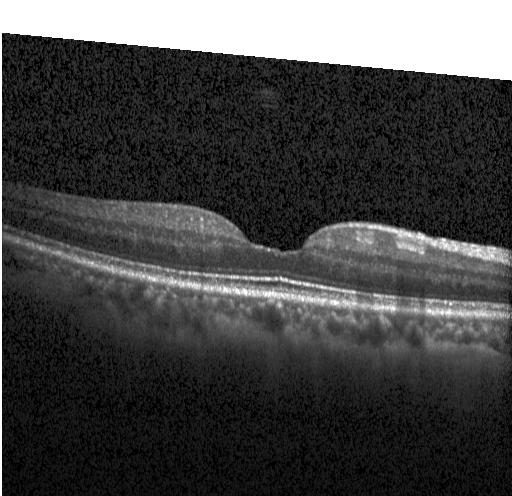

OCT finding: no choroidal neovascularization, no diabetic macular edema, and no drusen.